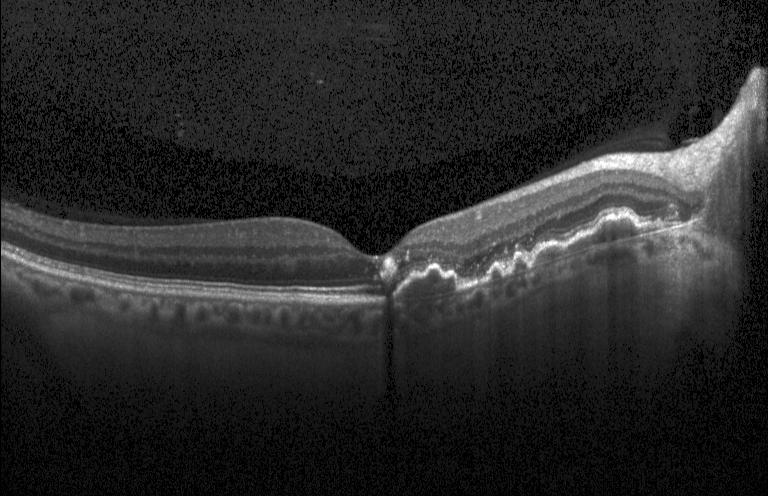 Spectral-domain OCT B-scan: CNV.